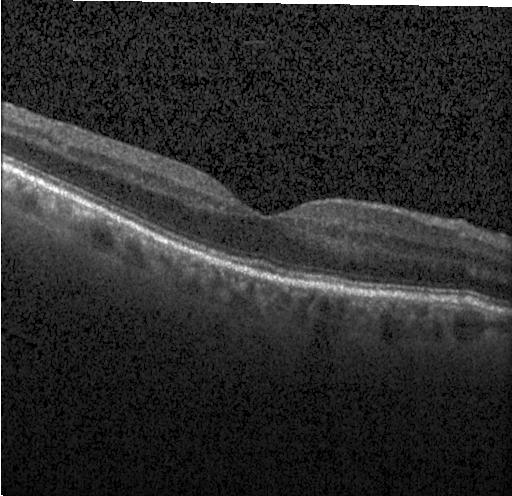
Finding: no evidence of choroidal neovascularization, diabetic macular edema, or drusen.